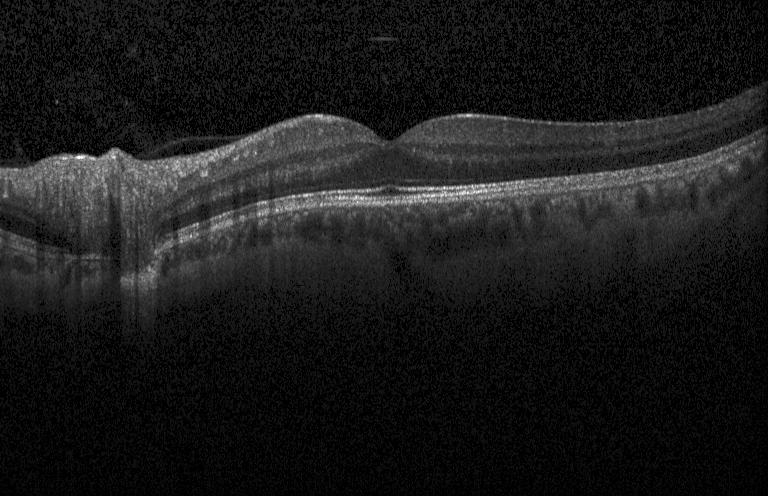 Horizontal scan through the fovea; optical coherence tomography B-scan; SD-OCT; Heidelberg Spectralis OCT system
Diagnosis: no choroidal neovascularization, no diabetic macular edema, and no drusen.